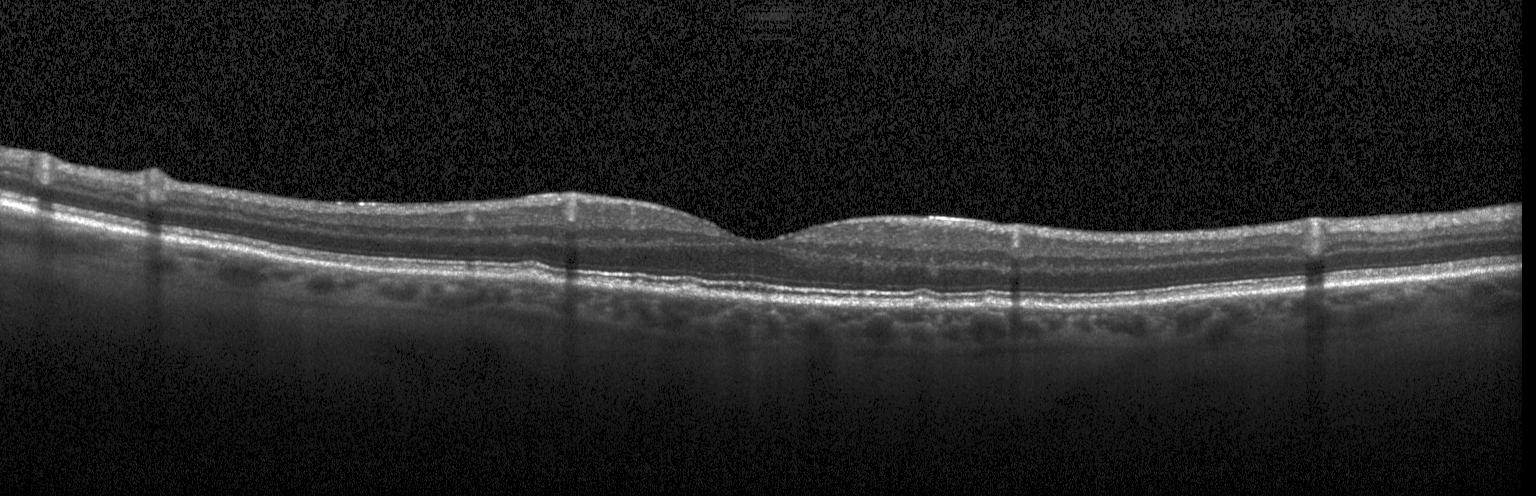

Heidelberg Spectralis, centered on the fovea, SD-OCT, retinal OCT B-scan
Assessment: sub-RPE drusenoid deposits.